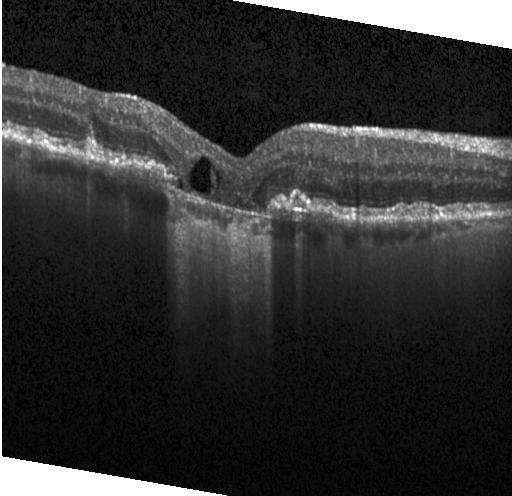
Fovea-centered · SD-OCT · acquired on a Heidelberg Spectralis · retinal OCT B-scan
Finding: CNV.